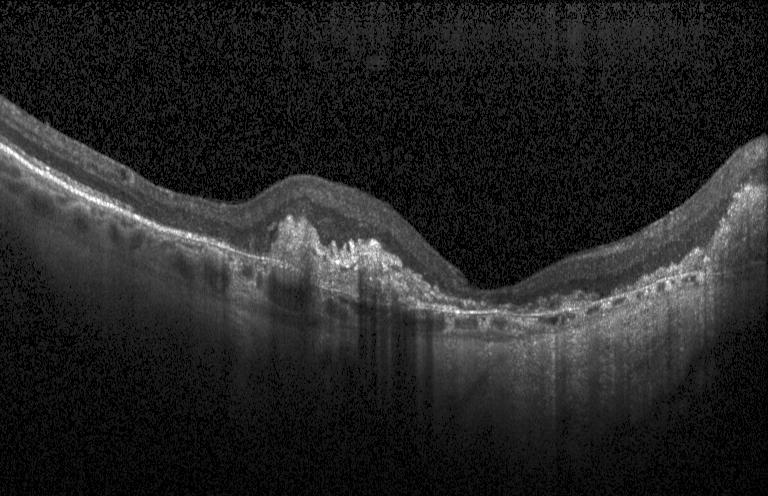
OCT B-scan · spectral-domain optical coherence tomography · Heidelberg Spectralis · centered on the fovea
Diagnosis: a choroidal neovascular membrane.